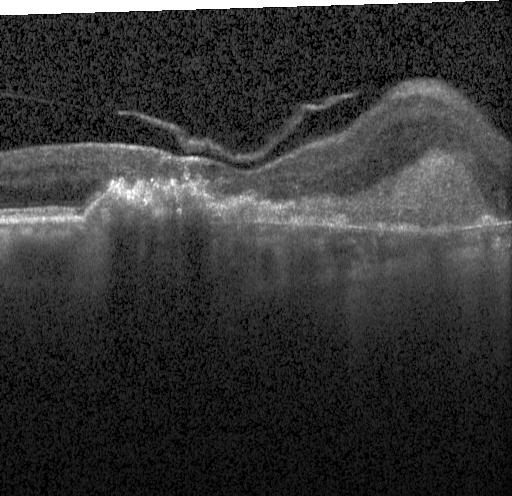

Macular OCT demonstrating CNV.